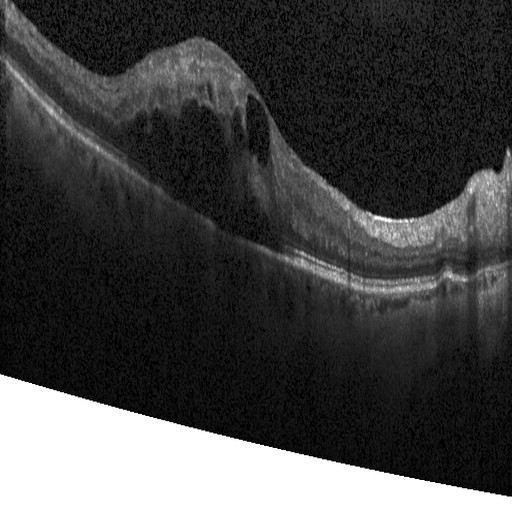 Acquired on a Heidelberg Spectralis. OCT line scan. Finding: diabetic macular edema (DME).